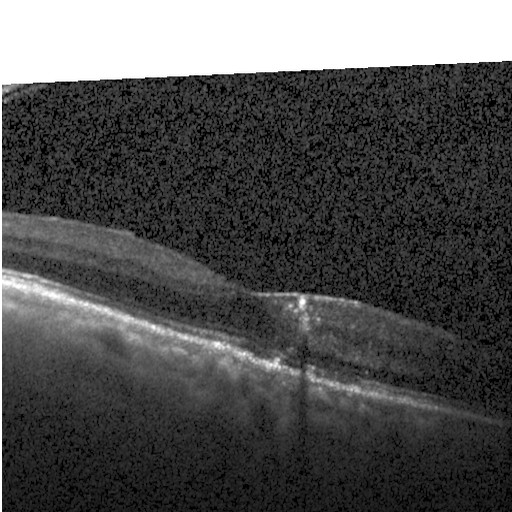 Finding: diabetic macular edema (DME).